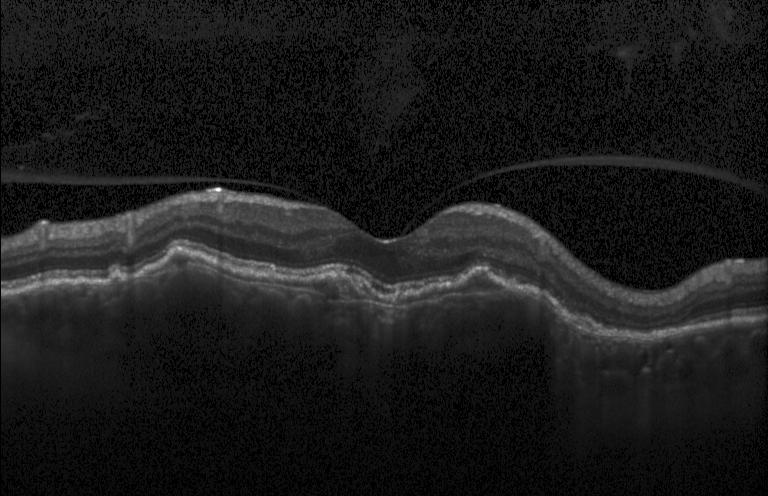

Optical coherence tomography B-scan
Dx: choroidal neovascularization (CNV).